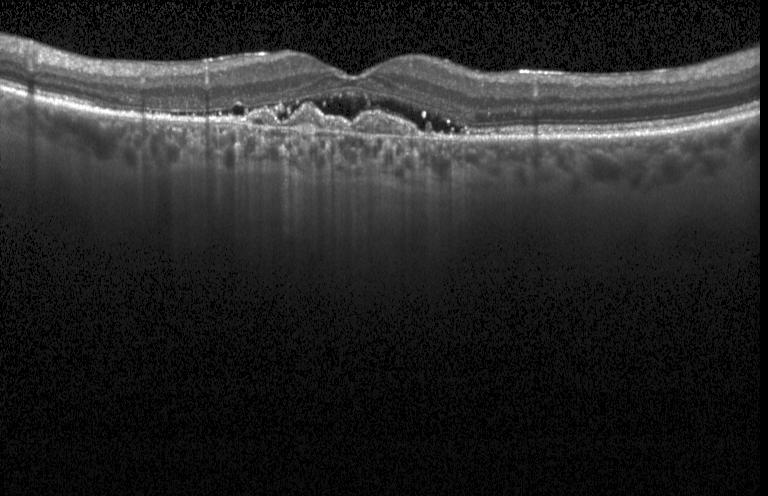 Retinal OCT B-scan. Acquired on a Heidelberg Spectralis
Finding: CNV.